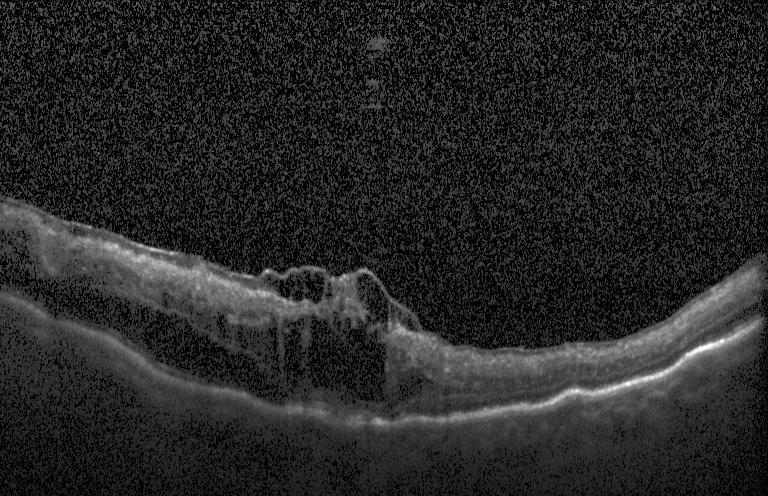

Acquired on a Heidelberg Spectralis · OCT line scan · spectral-domain OCT · horizontal scan through the fovea.
Diagnosis: DME.